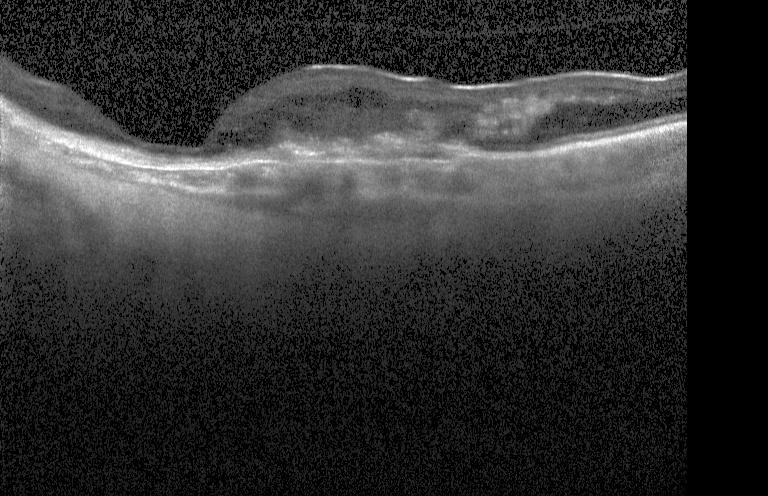

Spectral-domain OCT · acquired on a Heidelberg Spectralis · fovea-centered · retinal OCT B-scan
Assessment: a choroidal neovascular membrane.